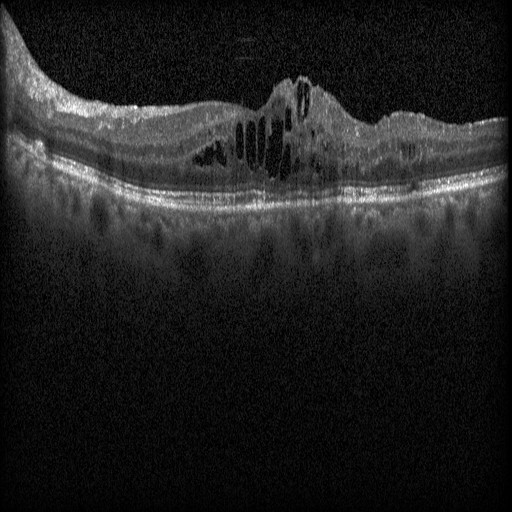

Macular OCT: diabetic macular edema.